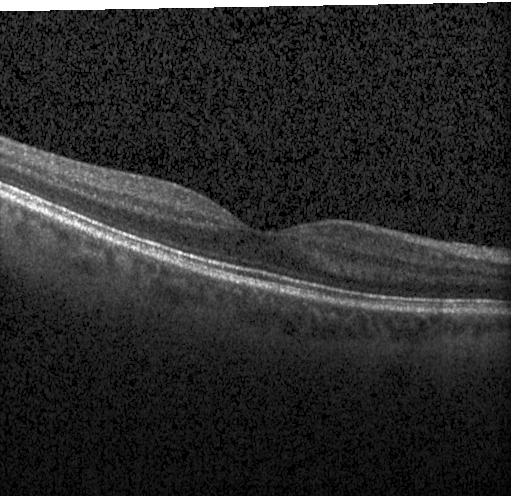 Diagnosis: no evidence of choroidal neovascularization, diabetic macular edema, or drusen.